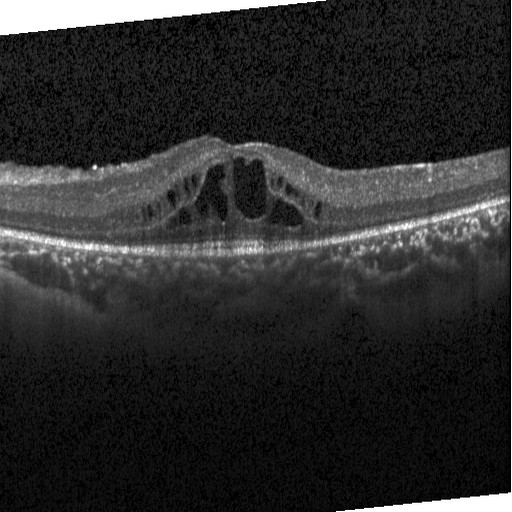
Macular OCT demonstrating DME.